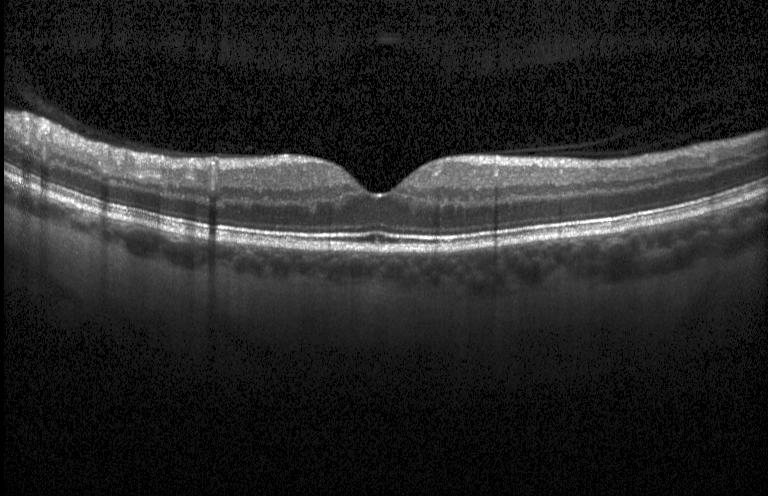

Retinal OCT cross-section — Impression: neither choroidal neovascularization, diabetic macular edema, nor drusen.